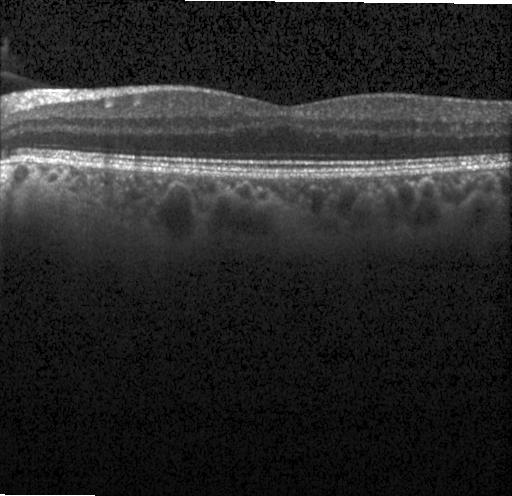

Macular OCT: no choroidal neovascularization, diabetic macular edema, or drusen.